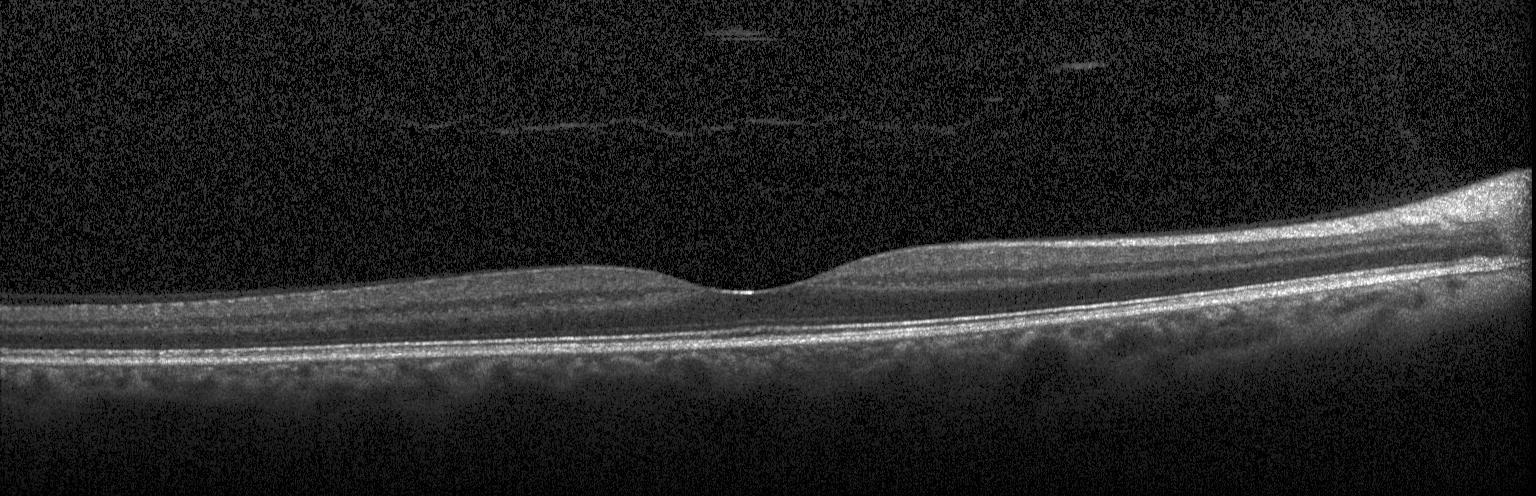

Diagnosis: no evidence of CNV, DME, or drusen.